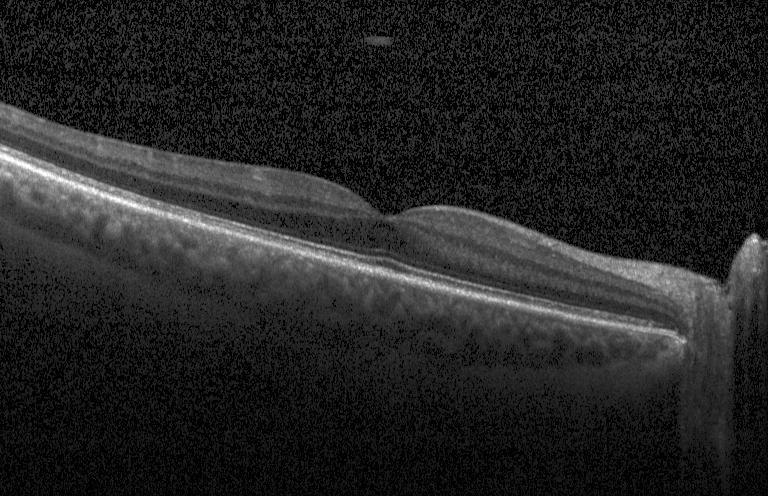

Macular scan, OCT B-scan, spectral-domain optical coherence tomography — The scan shows neither choroidal neovascularization, diabetic macular edema, nor drusen.